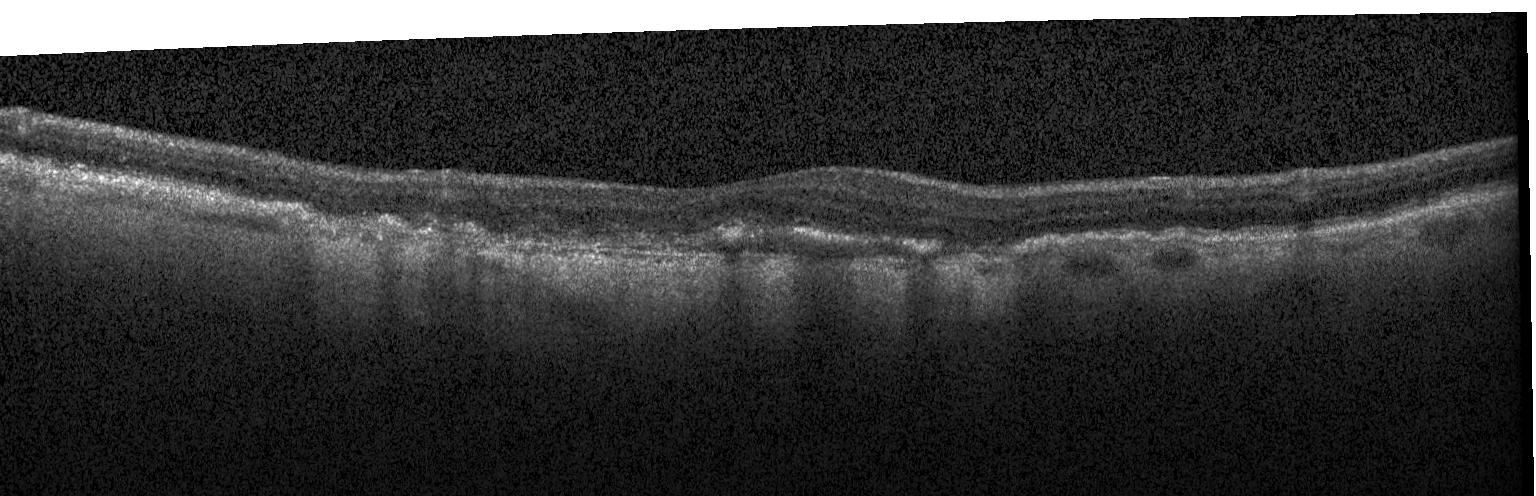
Instrument: Heidelberg Spectralis · OCT line scan — OCT finding: a choroidal neovascular membrane.